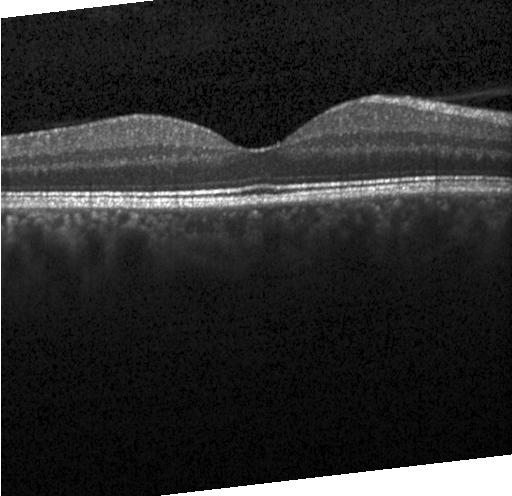 Optical coherence tomography scan. Spectral-domain OCT
No choroidal neovascularization, no diabetic macular edema, and no drusen.